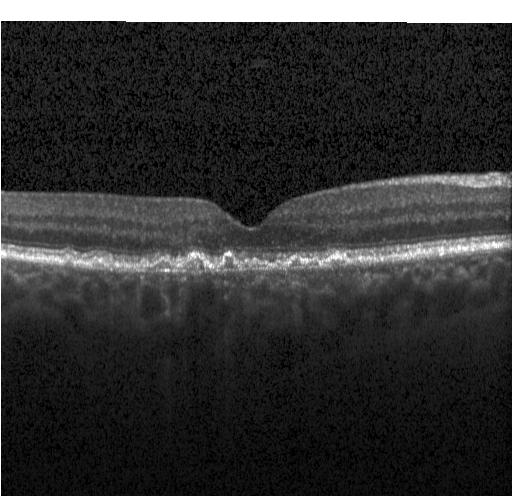 Retinal OCT cross-section. Instrument: Heidelberg Spectralis
Diagnosis: multiple drusen.